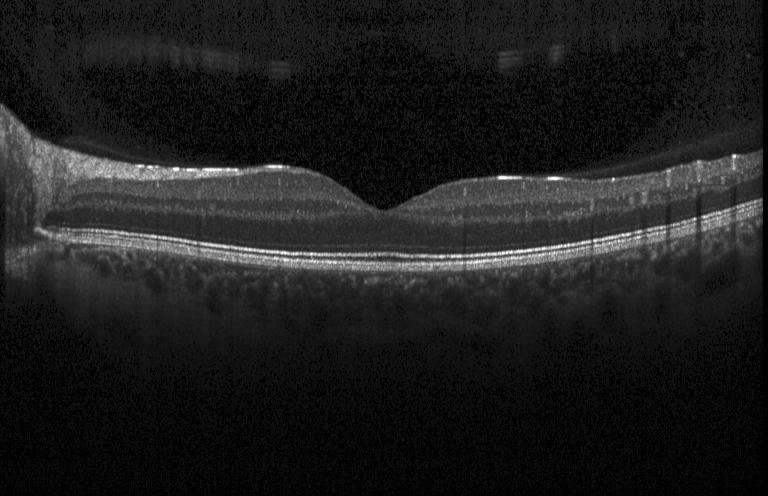
Diagnosis: neither choroidal neovascularization, diabetic macular edema, nor drusen.